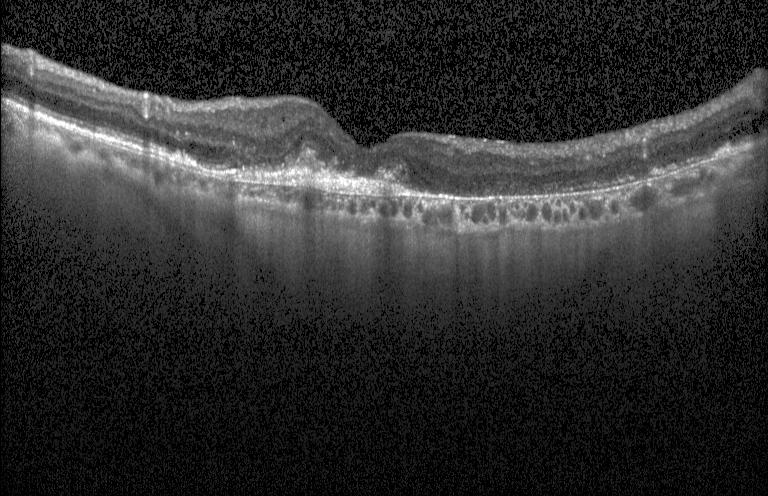
OCT line scan — OCT finding: choroidal neovascularization (CNV).